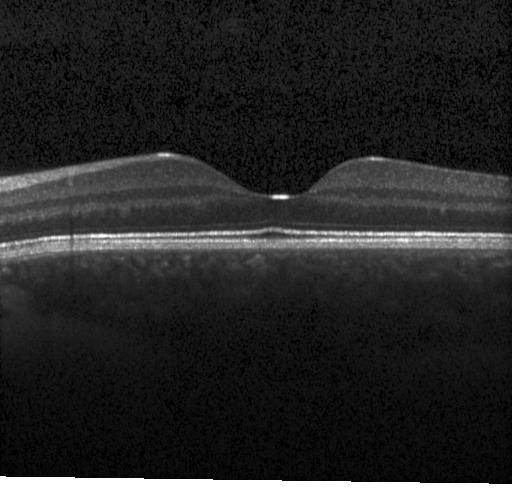 Optical coherence tomography scan — OCT finding: no choroidal neovascularization, diabetic macular edema, or drusen.